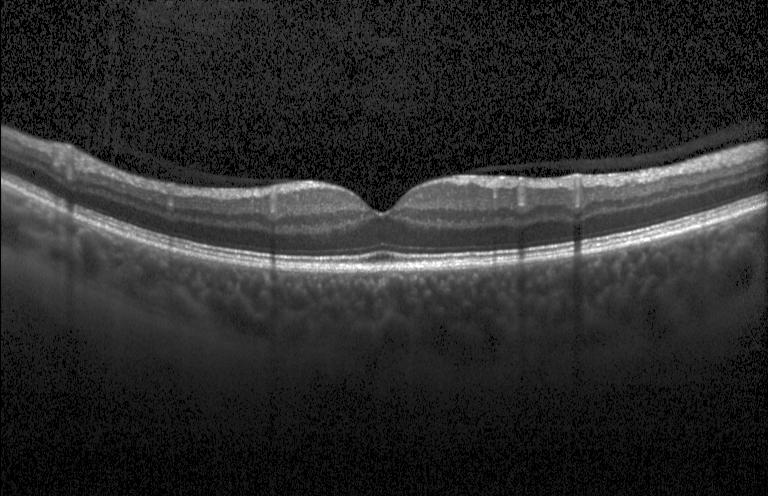
Impression: no evidence of CNV, DME, or drusen.